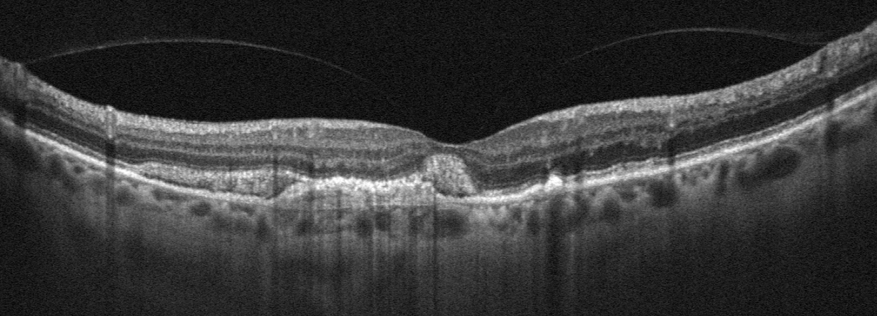

Retinal OCT cross-section.
OCT finding: AMD.